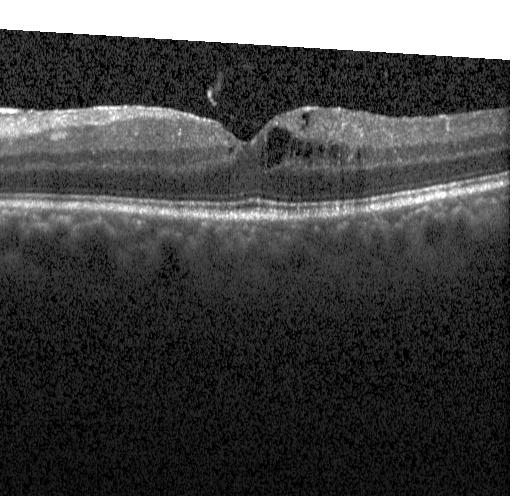 Retinal OCT cross-section; Heidelberg Spectralis OCT system; through the macula; spectral-domain optical coherence tomography.
Diagnosis: diabetic macular edema.